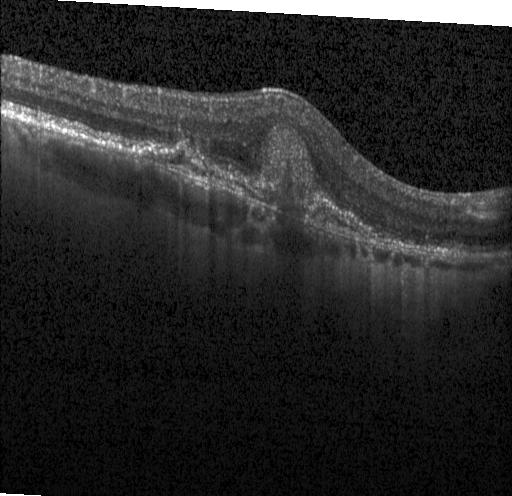 Retinal OCT B-scan. OCT finding: a choroidal neovascular membrane.